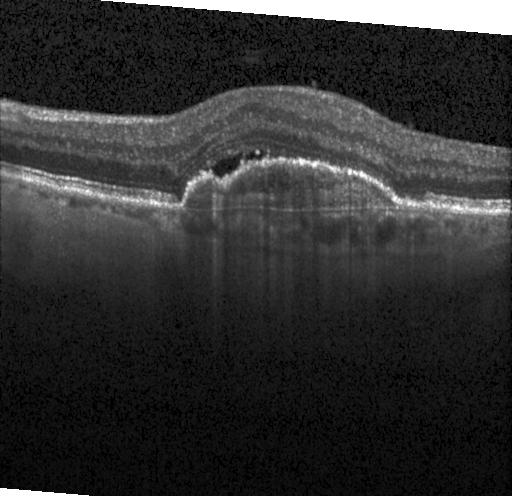 Finding: CNV.